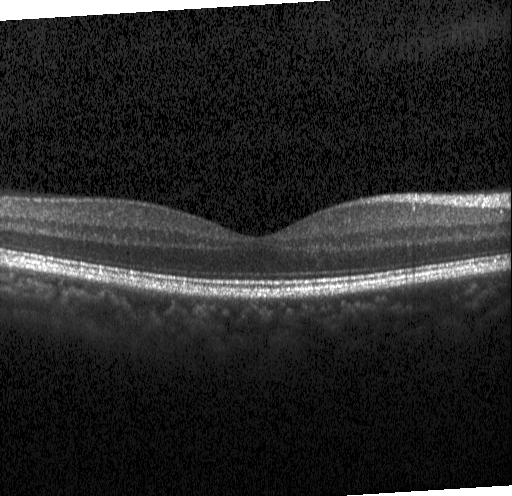 OCT B-scan showing no choroidal neovascularization, no diabetic macular edema, and no drusen.